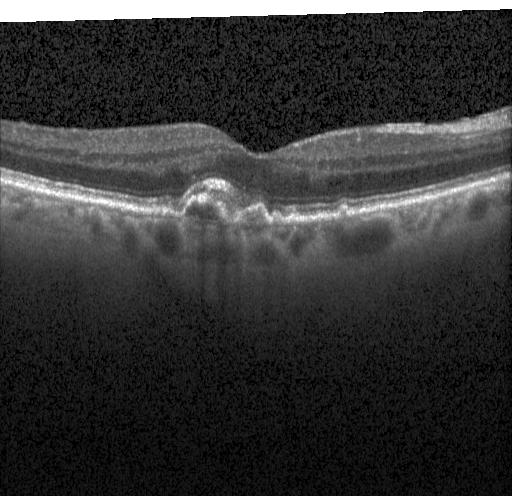

Macular OCT: a choroidal neovascular membrane.